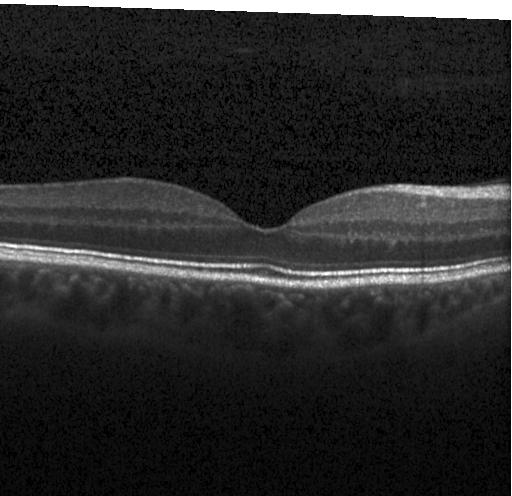 Optical coherence tomography scan.
Macular OCT: no choroidal neovascularization, no diabetic macular edema, and no drusen.